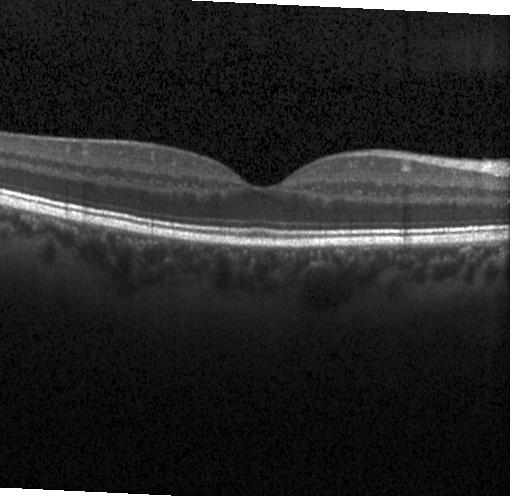 Acquired on a Heidelberg Spectralis, OCT line scan, spectral-domain OCT, through the macula.
Assessment: no choroidal neovascularization, diabetic macular edema, or drusen.